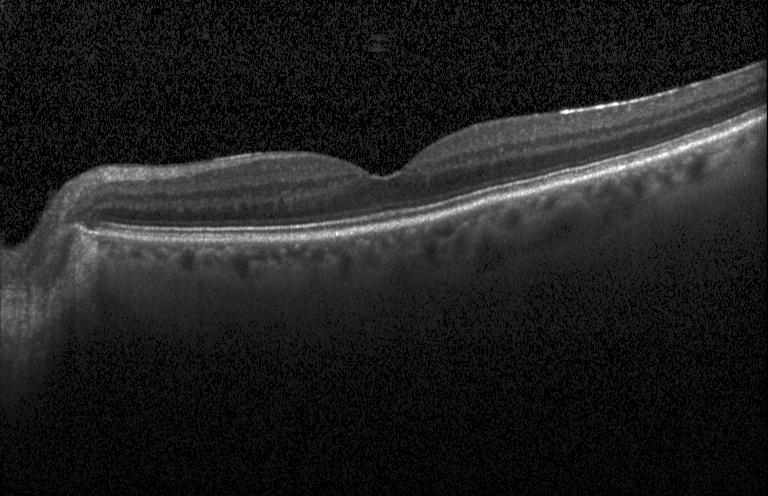 Retinal OCT B-scan — This B-scan demonstrates no evidence of choroidal neovascularization, diabetic macular edema, or drusen.